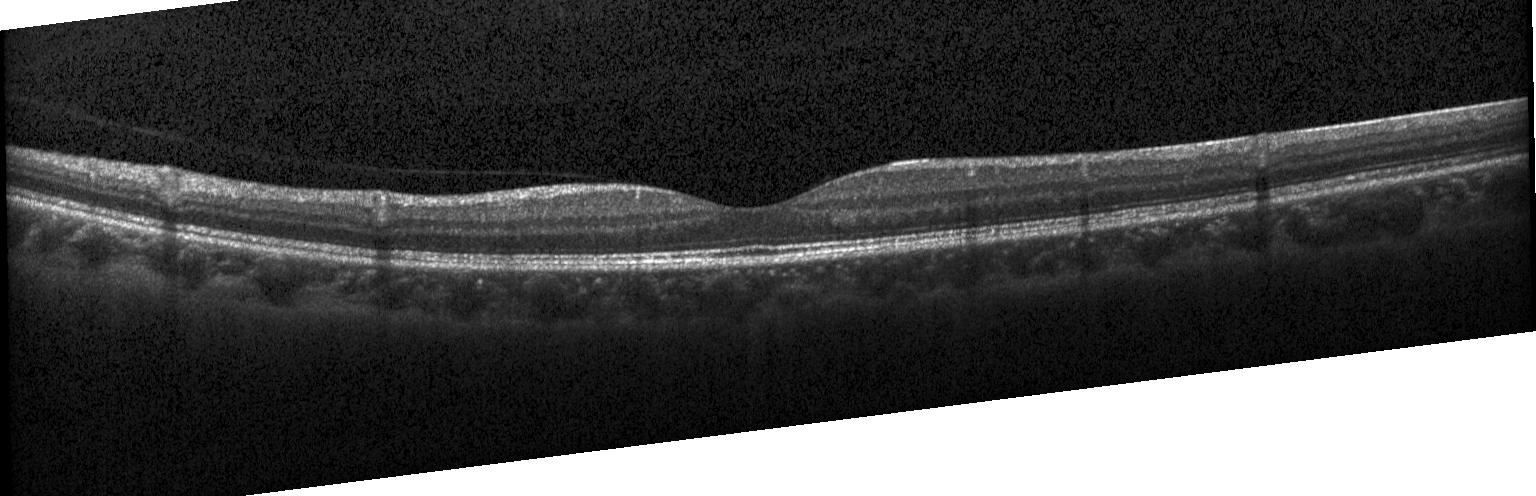

Spectral-domain OCT B-scan: neither CNV, DME, nor drusen.